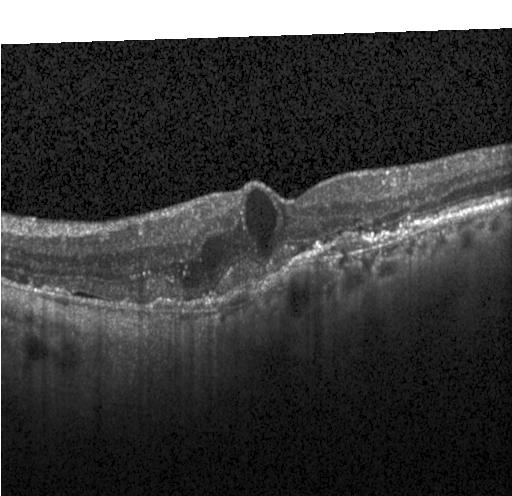
Spectral-domain OCT B-scan: a choroidal neovascular membrane.